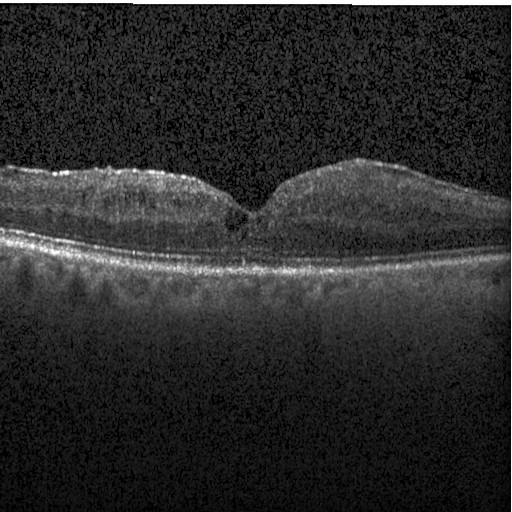

Impression: DME.